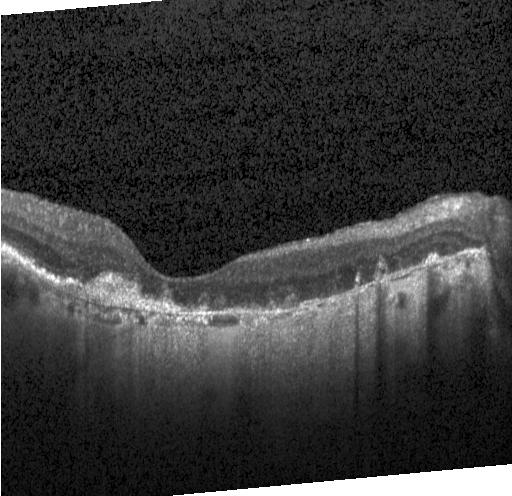 Finding: a choroidal neovascular membrane.